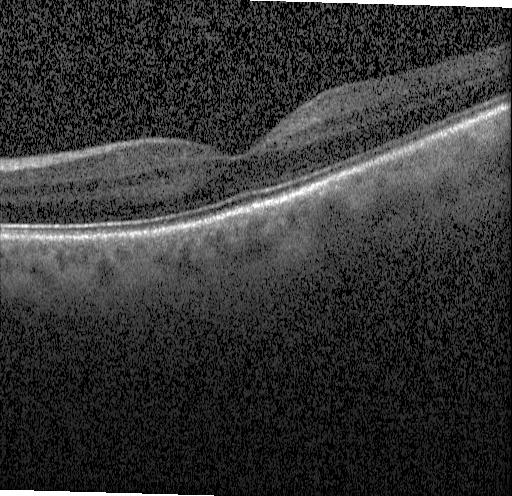 Retinal OCT B-scan · horizontal scan through the fovea · acquired on a Heidelberg Spectralis.
The scan shows no evidence of CNV, DME, or drusen.